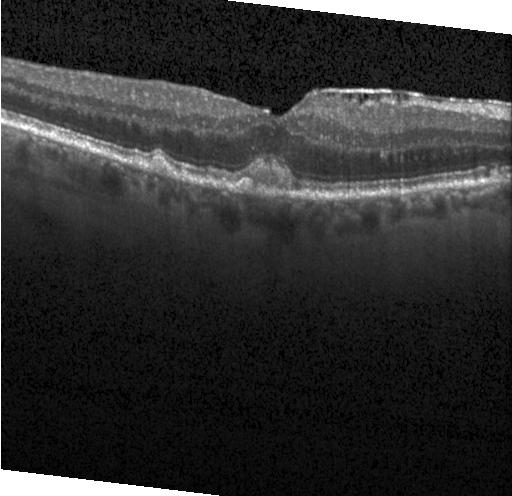 Drusen.